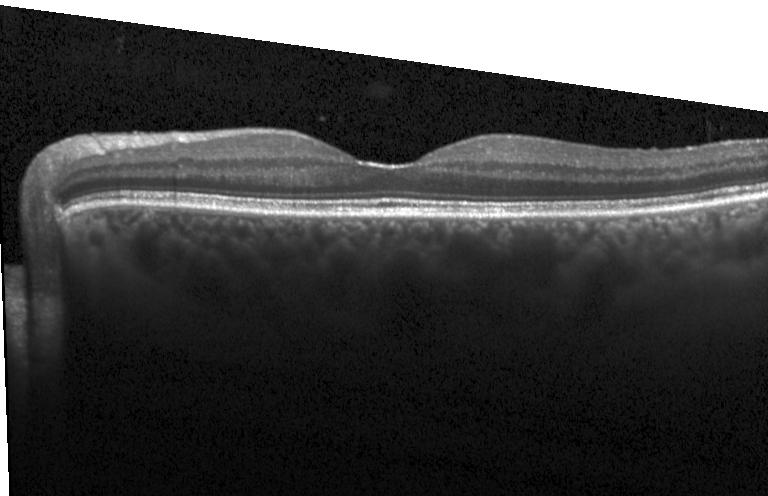 Optical coherence tomography scan, Heidelberg Spectralis, fovea-centered. This B-scan demonstrates no CNV, DME, or drusen.